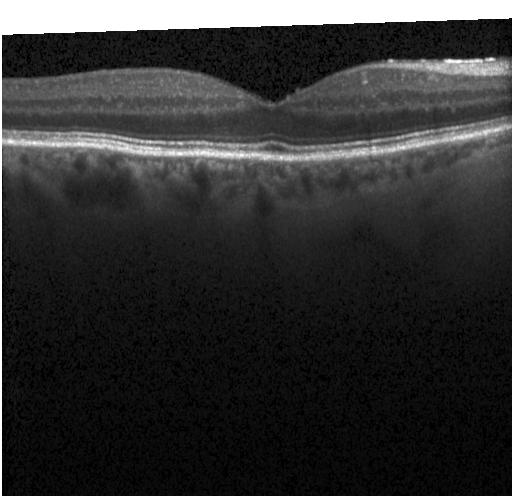
Acquired on a Heidelberg Spectralis. Retinal OCT cross-section — Diagnosis: no choroidal neovascularization, no diabetic macular edema, and no drusen.